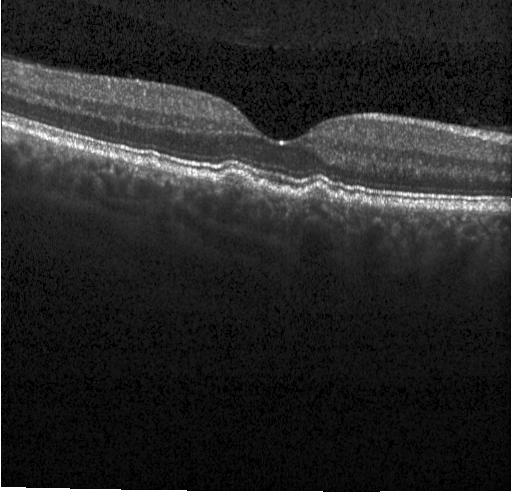

Retinal OCT cross-section showing multiple drusen.